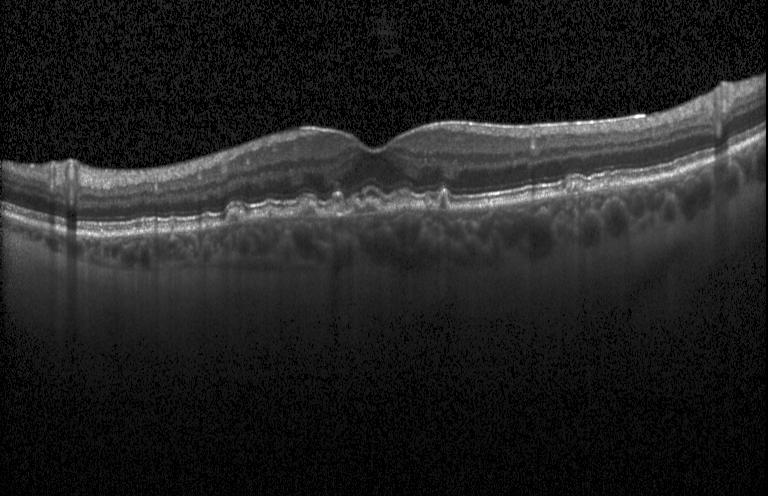

Spectral-domain OCT B-scan: sub-RPE drusenoid deposits.